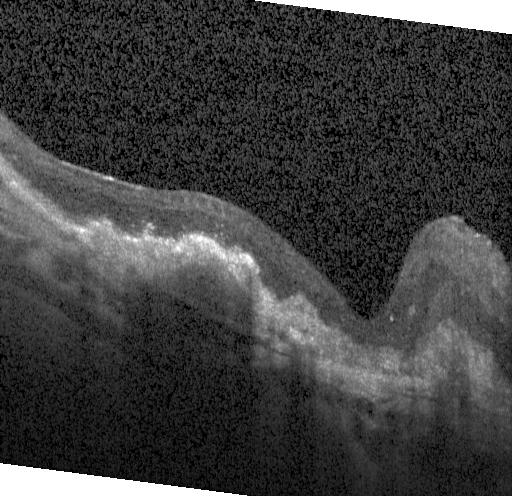
Optical coherence tomography B-scan. Impression: a choroidal neovascular membrane.